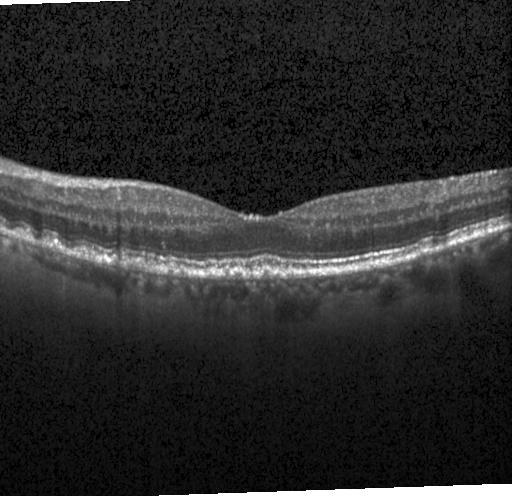
Macular OCT: multiple drusen.